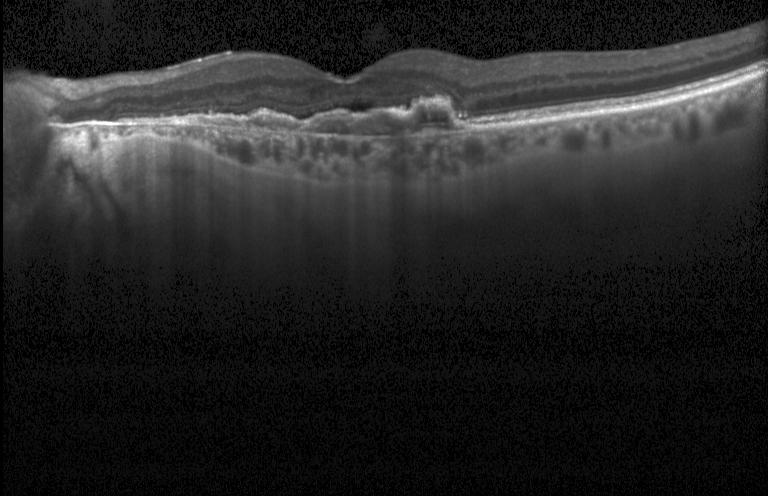 Heidelberg Spectralis, OCT B-scan
Dx: choroidal neovascularization (CNV).